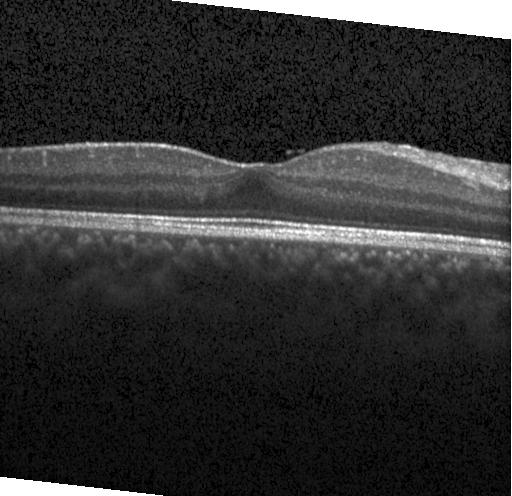 Diagnosis: no evidence of CNV, DME, or drusen.